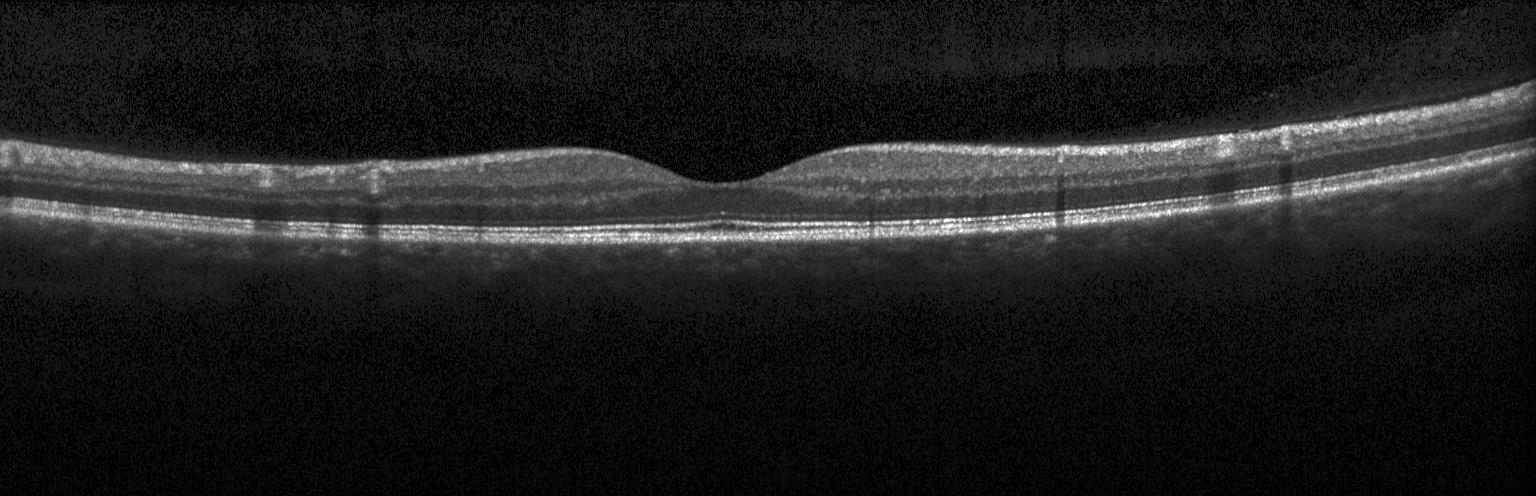
Diagnosis: no evidence of choroidal neovascularization, diabetic macular edema, or drusen.